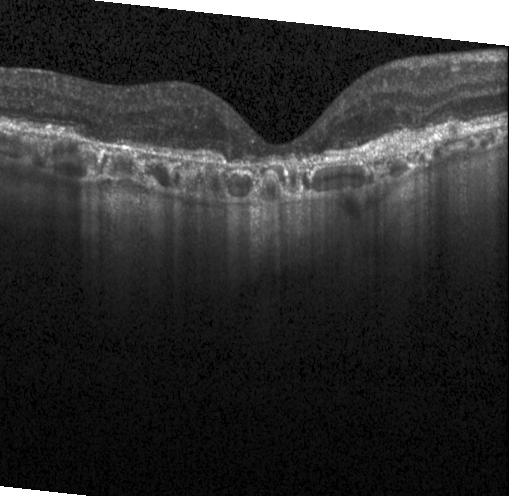

Impression: a choroidal neovascular membrane.